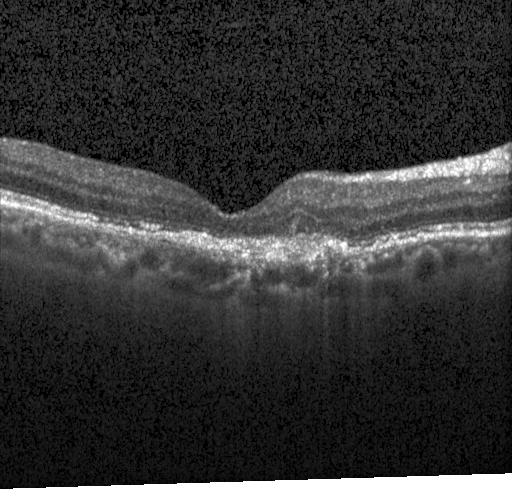 OCT scan showing choroidal neovascularization.